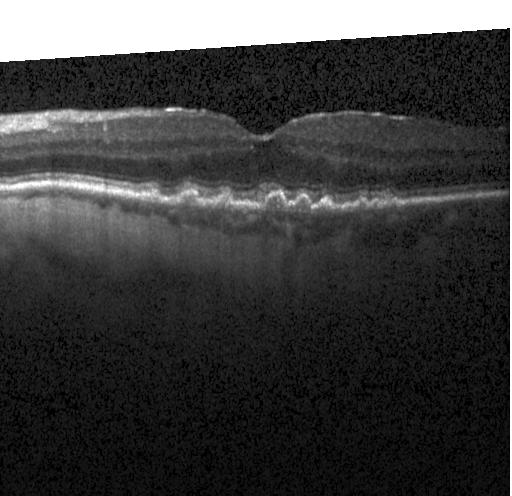

OCT B-scan showing sub-RPE drusenoid deposits.